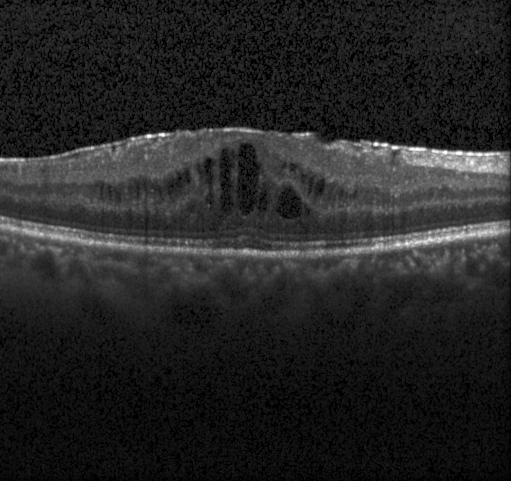

Retinal OCT cross-section. Finding: DME.